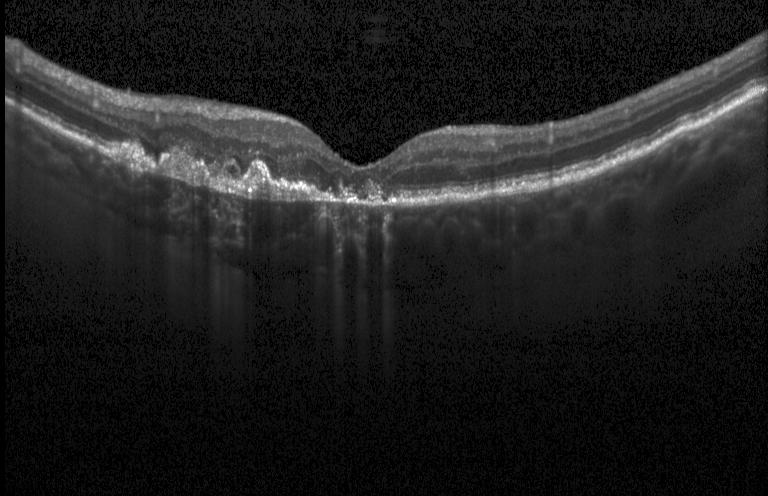 Instrument: Heidelberg Spectralis · optical coherence tomography B-scan.
CNV.